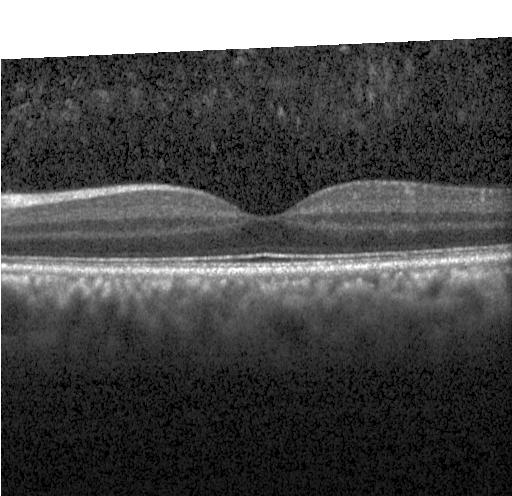

Dx: neither CNV, DME, nor drusen.